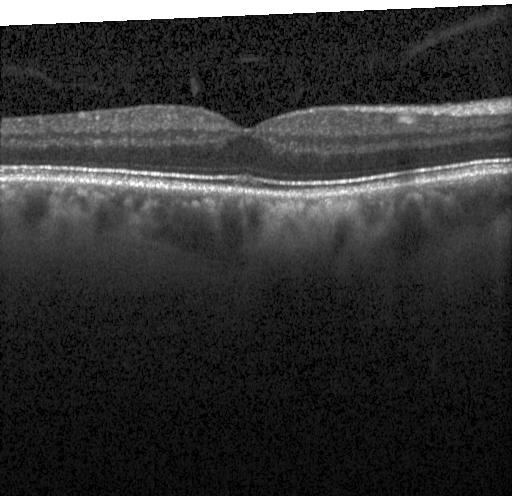 OCT finding: no evidence of choroidal neovascularization, diabetic macular edema, or drusen.